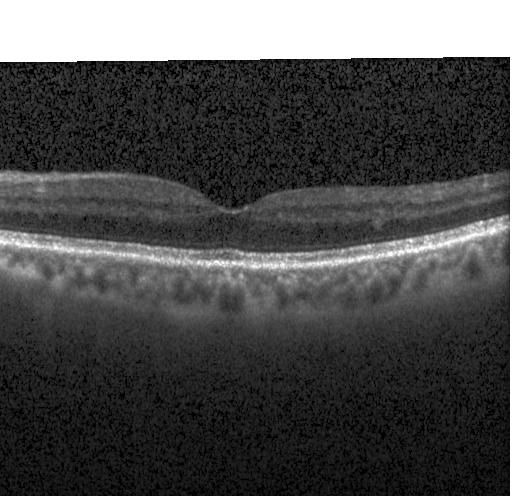 Spectral-domain optical coherence tomography; Heidelberg Spectralis OCT system; OCT B-scan; fovea-centered
The scan shows no choroidal neovascularization, no diabetic macular edema, and no drusen.